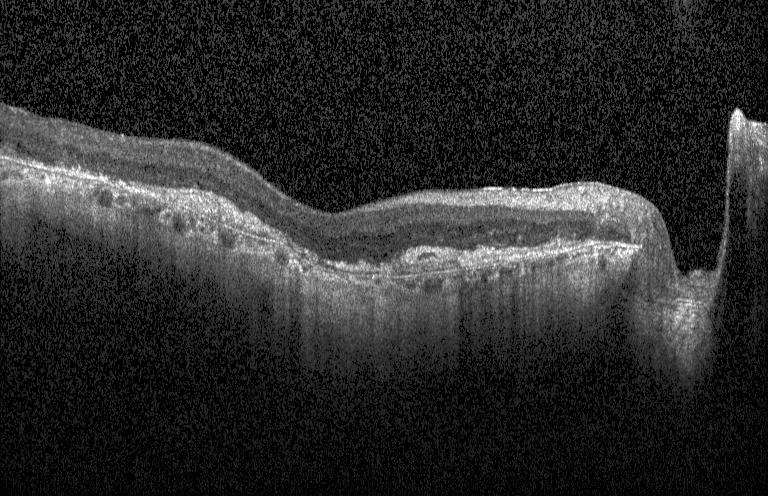 Spectral-domain OCT. Heidelberg Spectralis OCT system. OCT B-scan. Macular scan
Diagnosis: CNV.